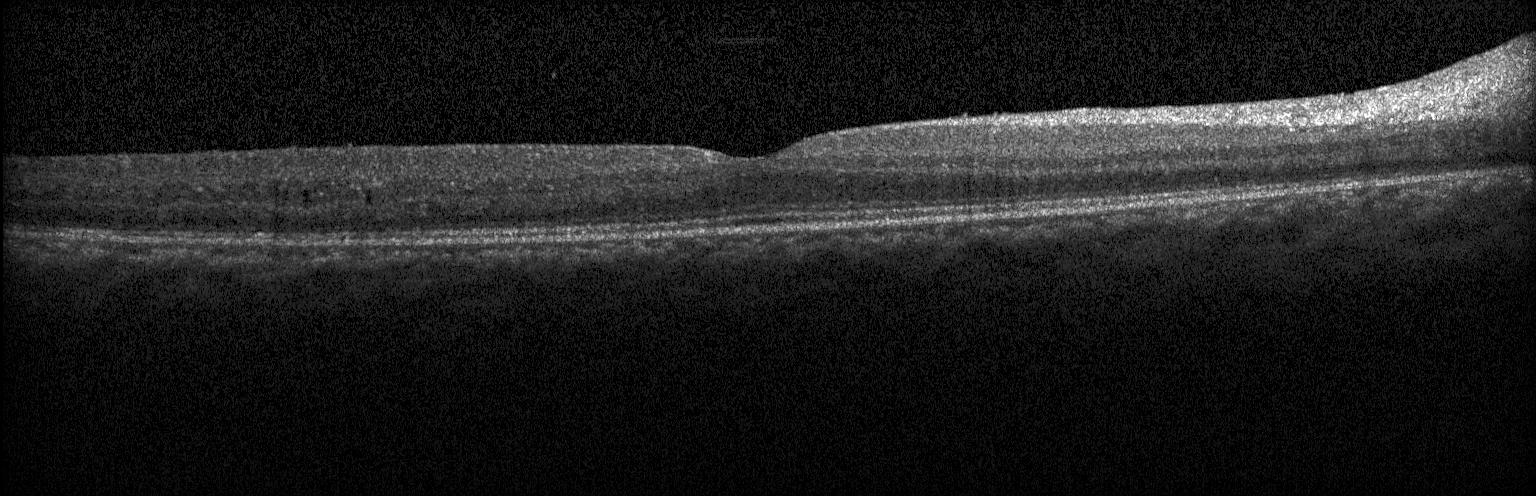

Centered on the fovea · optical coherence tomography scan — Finding: DME.